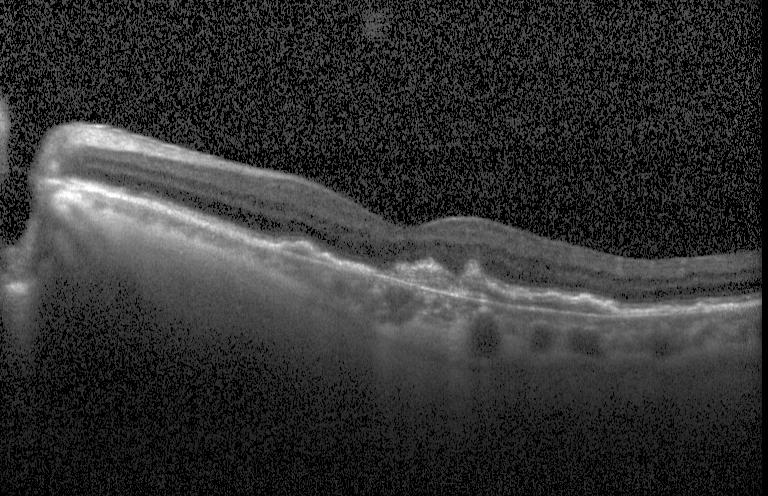

OCT B-scan showing a choroidal neovascular membrane.